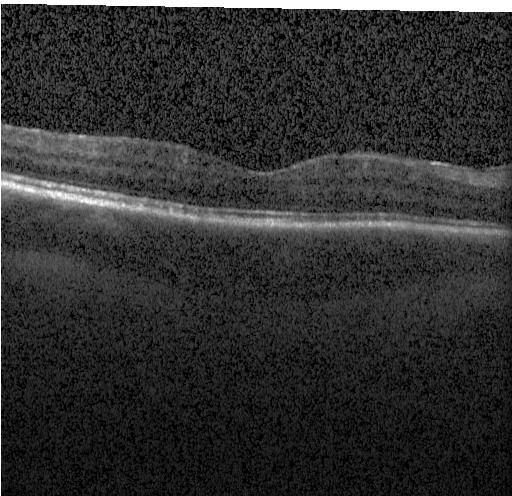
Optical coherence tomography B-scan; fovea-centered; spectral-domain OCT. Impression: no choroidal neovascularization, no diabetic macular edema, and no drusen.